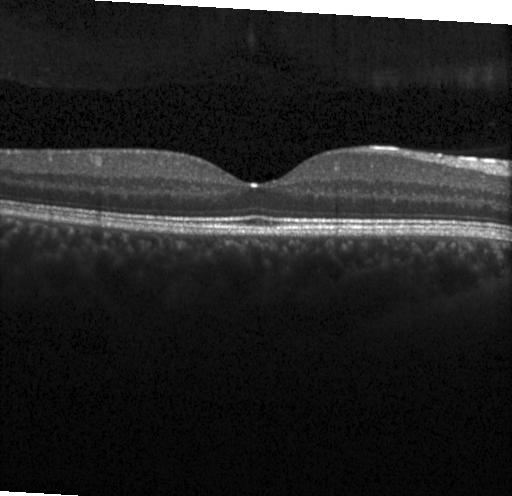 Optical coherence tomography scan. Impression: neither choroidal neovascularization, diabetic macular edema, nor drusen.